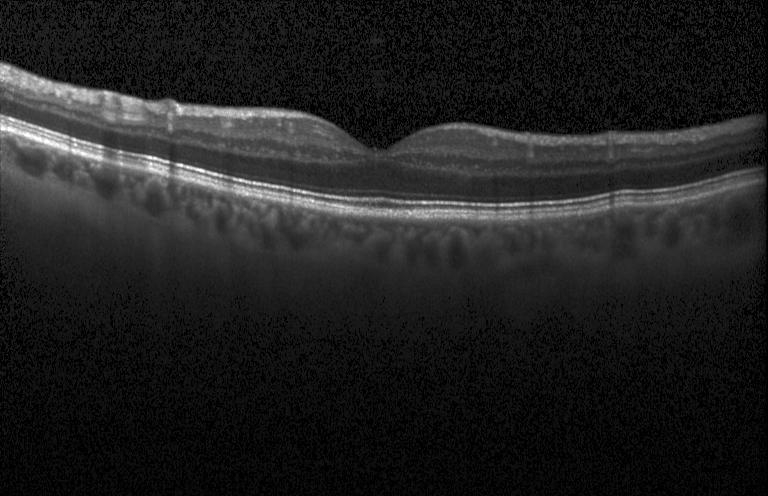 Heidelberg Spectralis · retinal OCT B-scan · SD-OCT · horizontal scan through the fovea. Macular OCT: no choroidal neovascularization, diabetic macular edema, or drusen.